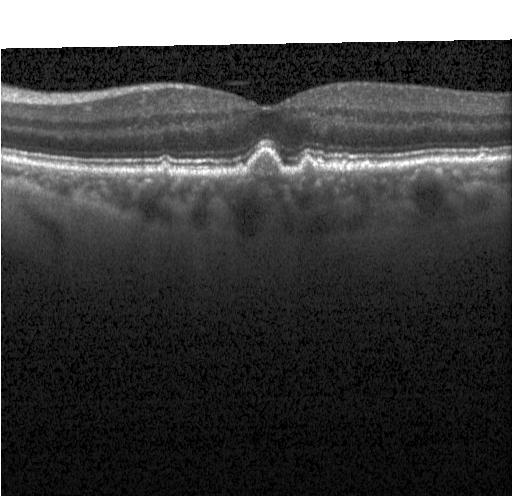

Acquired on a Heidelberg Spectralis; retinal OCT B-scan; horizontal scan through the fovea
Finding: multiple drusen.